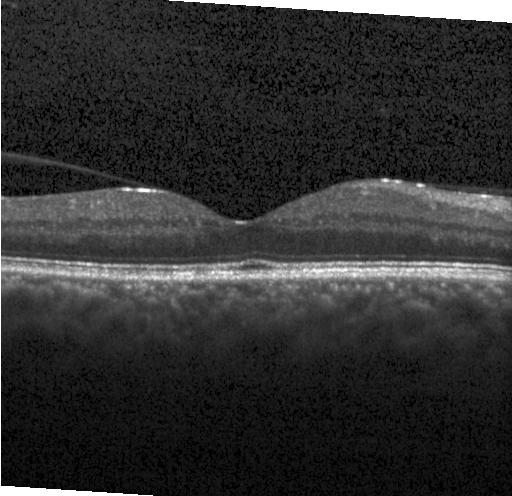

OCT B-scan showing no choroidal neovascularization, diabetic macular edema, or drusen.